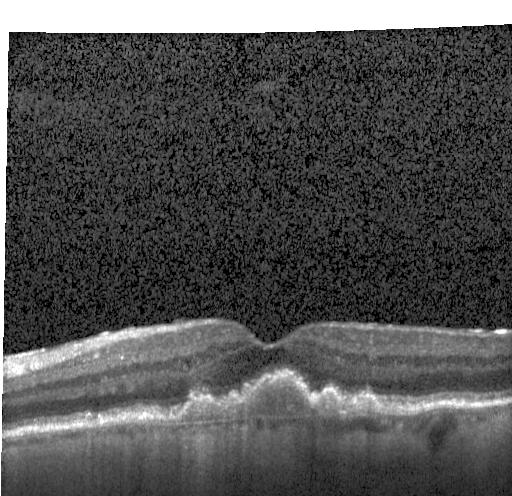 Assessment: a choroidal neovascular membrane.